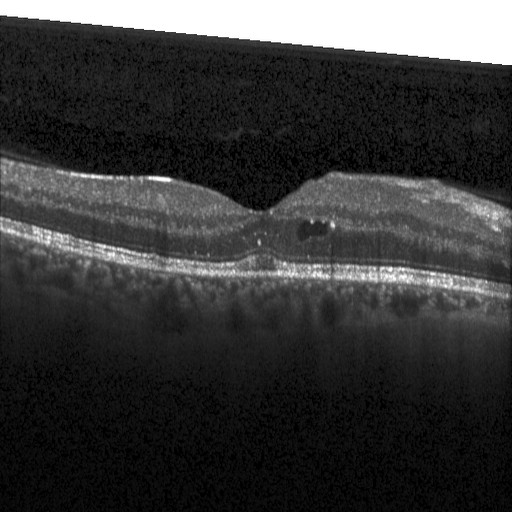

Assessment: diabetic macular edema.